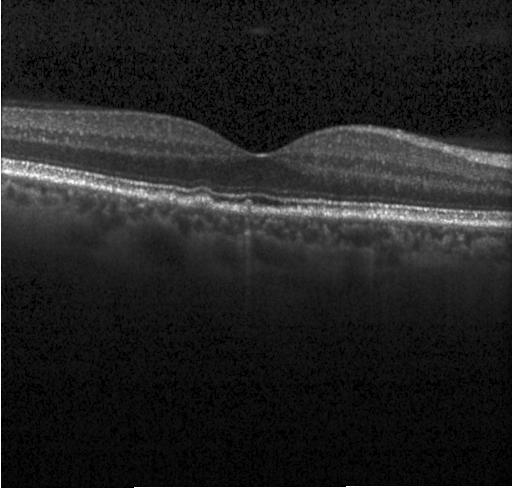 Retinal OCT cross-section, Heidelberg Spectralis, SD-OCT, macular scan. OCT finding: drusen.